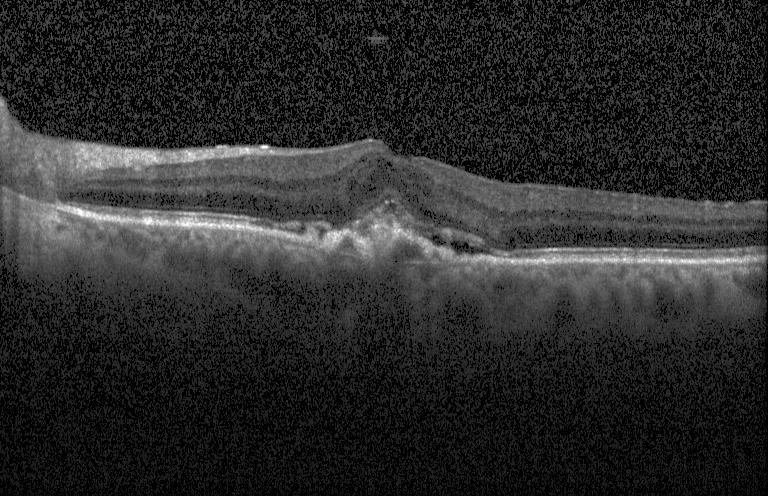 Optical coherence tomography B-scan · SD-OCT
Impression: a choroidal neovascular membrane.